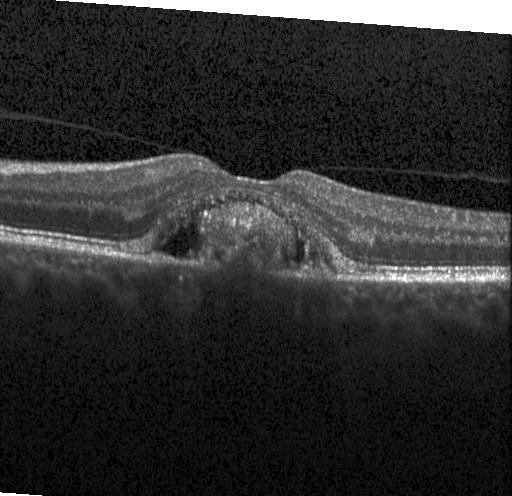
OCT line scan, acquired on a Heidelberg Spectralis — The scan shows choroidal neovascularization.